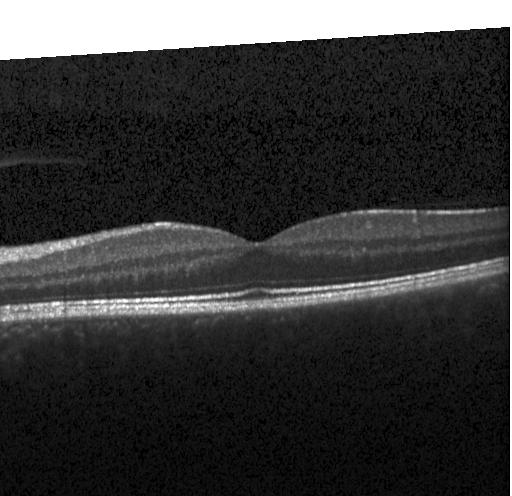

Retinal OCT cross-section; SD-OCT
Diagnosis: neither CNV, DME, nor drusen.